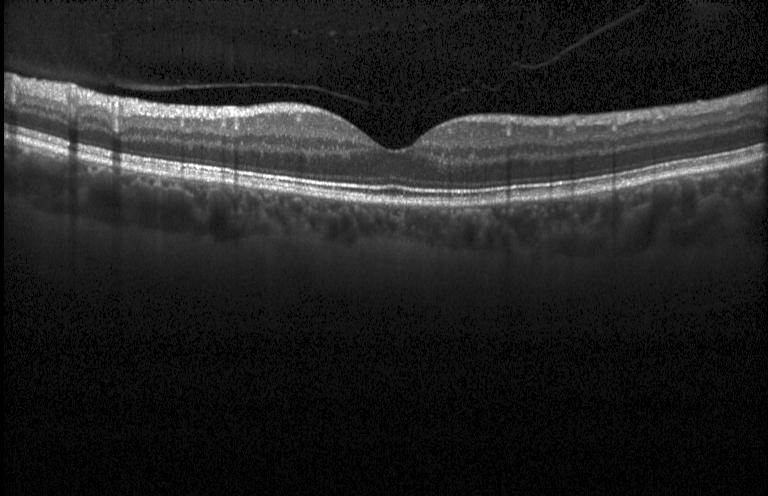
Optical coherence tomography scan; instrument: Heidelberg Spectralis.
No CNV, DME, or drusen.